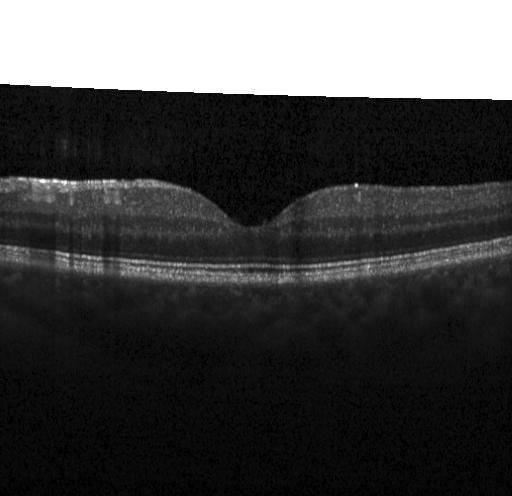

Optical coherence tomography scan; acquired on a Heidelberg Spectralis; macular scan; spectral-domain optical coherence tomography
Dx: no evidence of choroidal neovascularization, diabetic macular edema, or drusen.